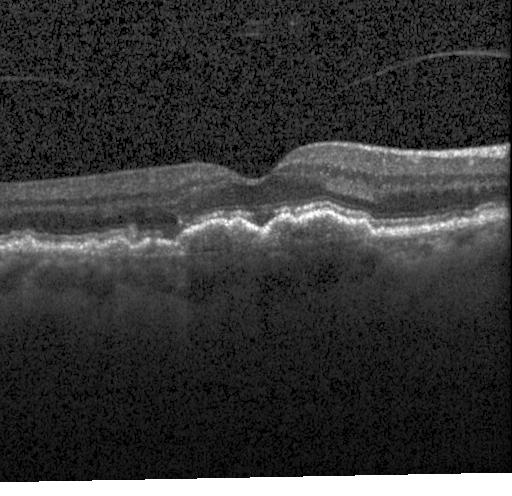

Spectral-domain OCT B-scan: choroidal neovascularization (CNV).